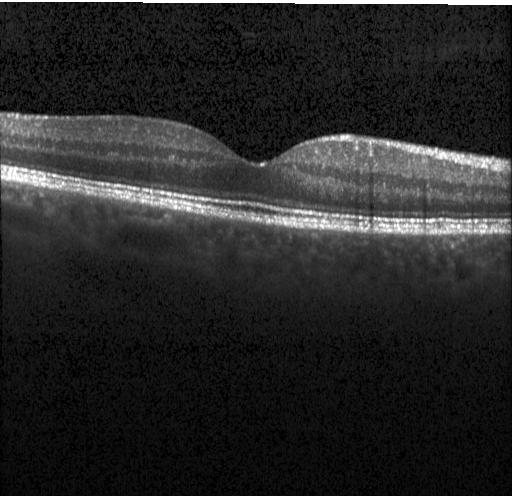 Optical coherence tomography scan, centered on the fovea.
Diagnosis: no evidence of choroidal neovascularization, diabetic macular edema, or drusen.